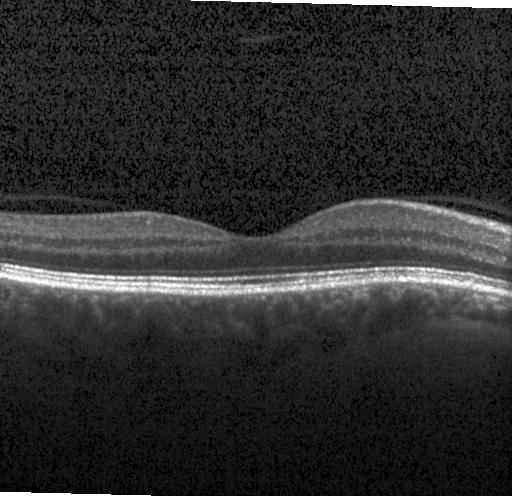
Impression: no choroidal neovascularization, no diabetic macular edema, and no drusen.